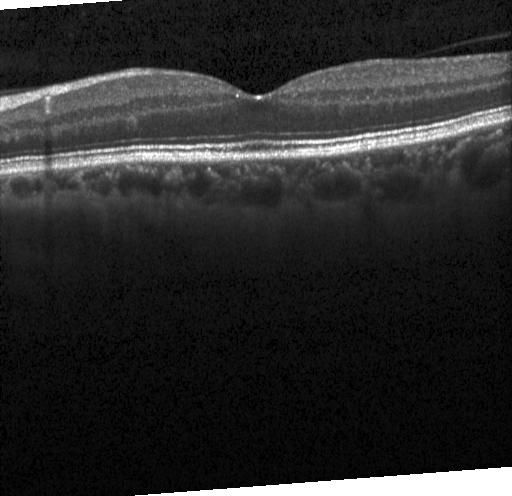 No CNV, DME, or drusen.